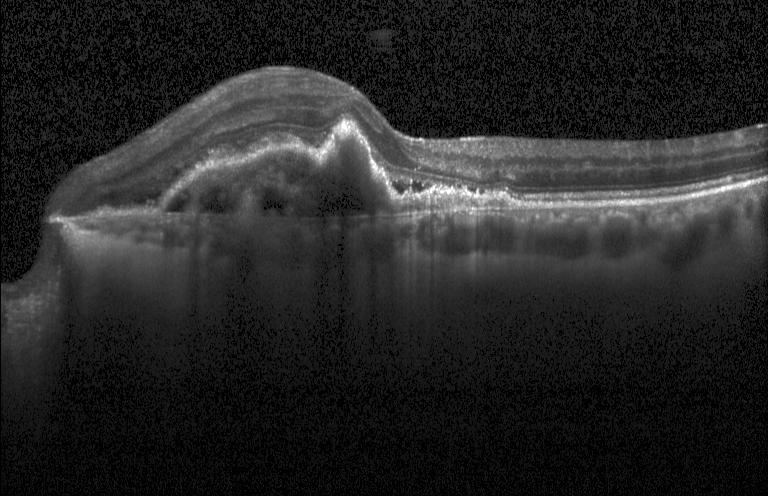

Macular OCT: a choroidal neovascular membrane.